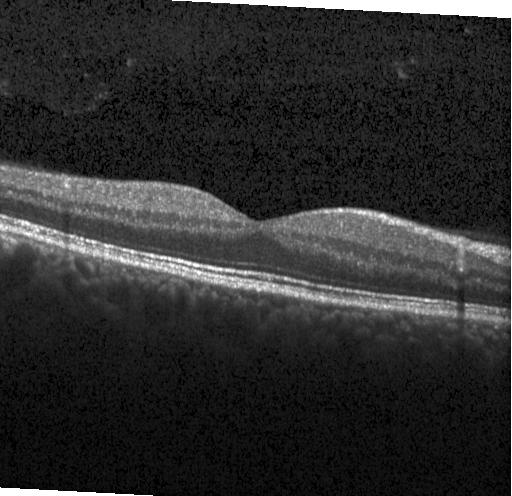

No CNV, no DME, and no drusen.